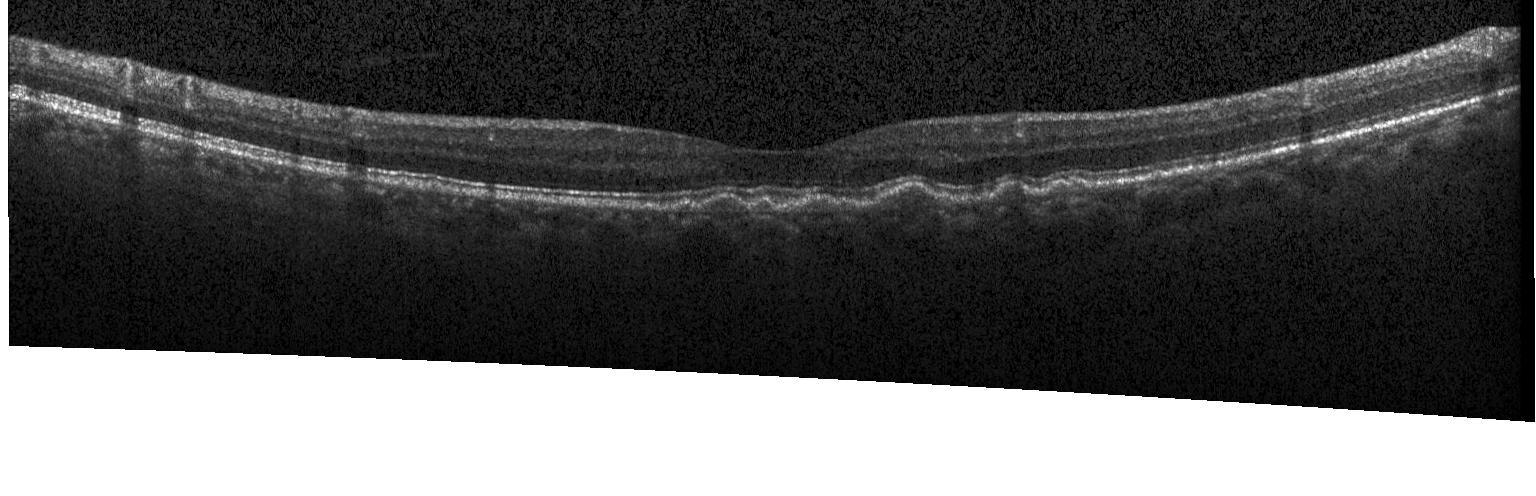 Heidelberg Spectralis, optical coherence tomography scan, horizontal scan through the fovea
Diagnosis: multiple drusen.